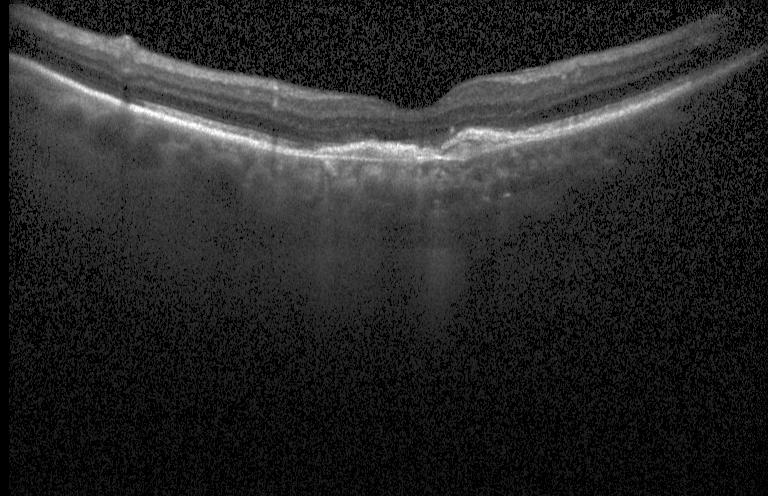

OCT B-scan — Finding: choroidal neovascularization (CNV).